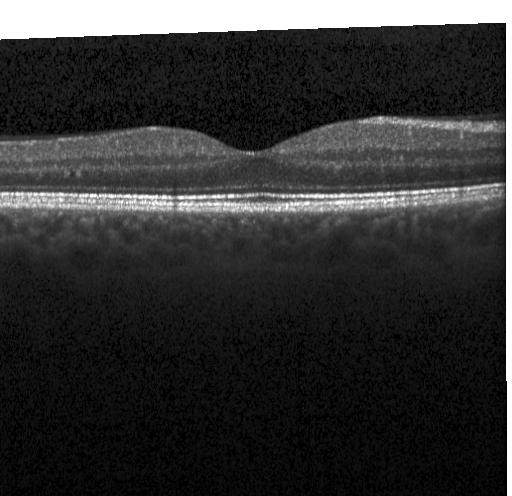

Centered on the fovea. SD-OCT. Instrument: Heidelberg Spectralis. OCT B-scan — The scan shows no choroidal neovascularization, diabetic macular edema, or drusen.